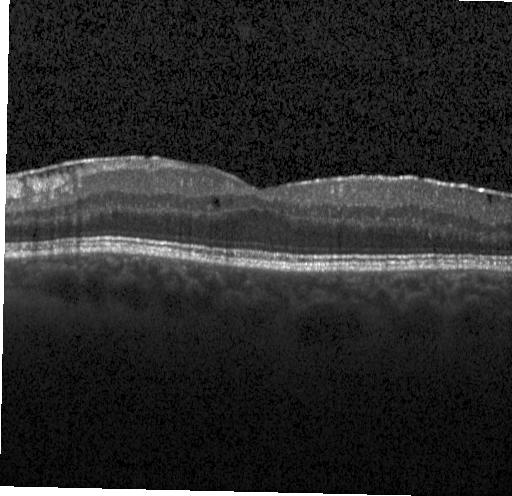 OCT scan showing DME.